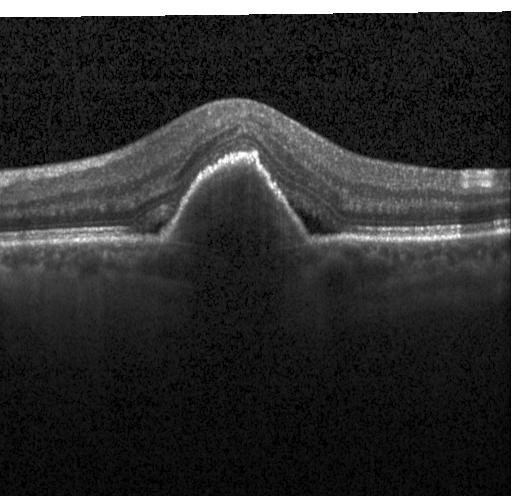 Optical coherence tomography scan.
OCT finding: CNV.